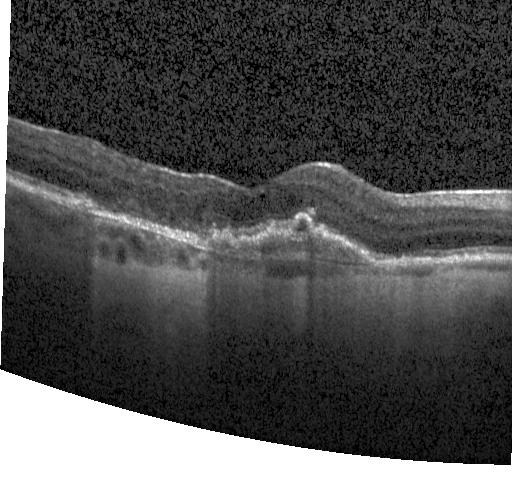

Through the macula; OCT B-scan
The scan shows CNV.